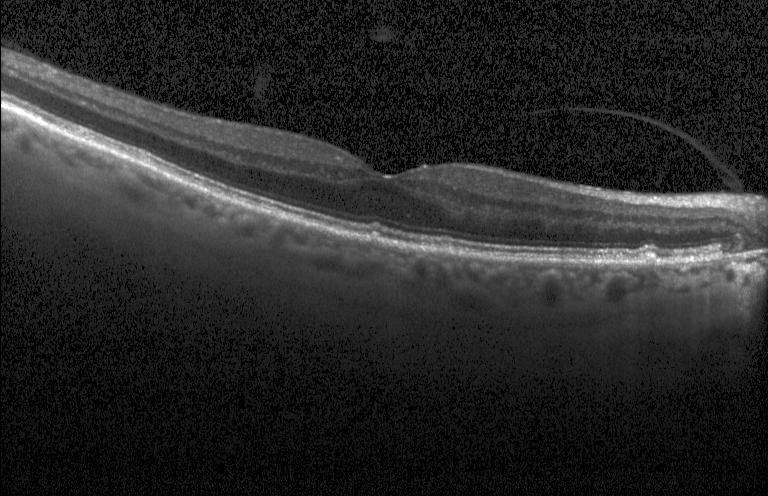
OCT B-scan showing no choroidal neovascularization, diabetic macular edema, or drusen.